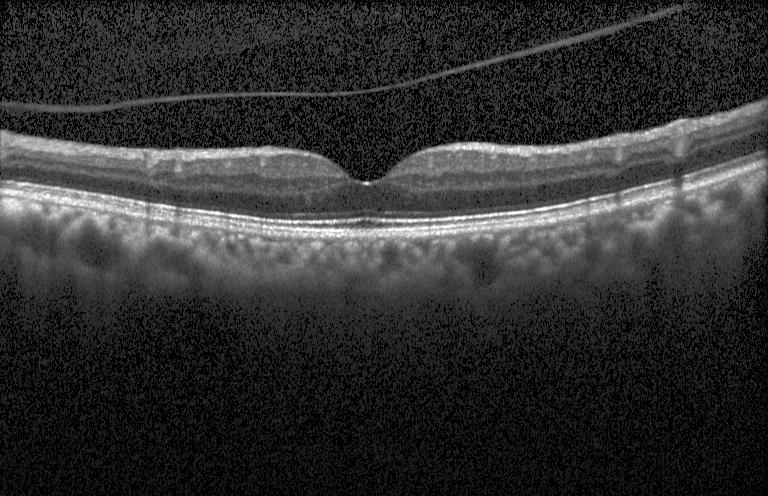
Optical coherence tomography B-scan, spectral-domain OCT, fovea-centered, acquired on a Heidelberg Spectralis — Finding: no choroidal neovascularization, no diabetic macular edema, and no drusen.